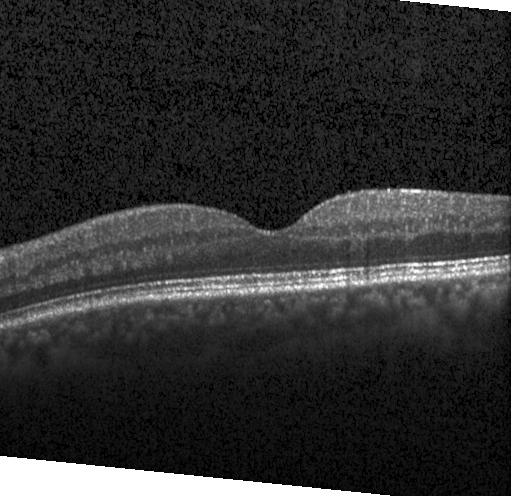

SD-OCT, optical coherence tomography scan.
OCT finding: neither choroidal neovascularization, diabetic macular edema, nor drusen.